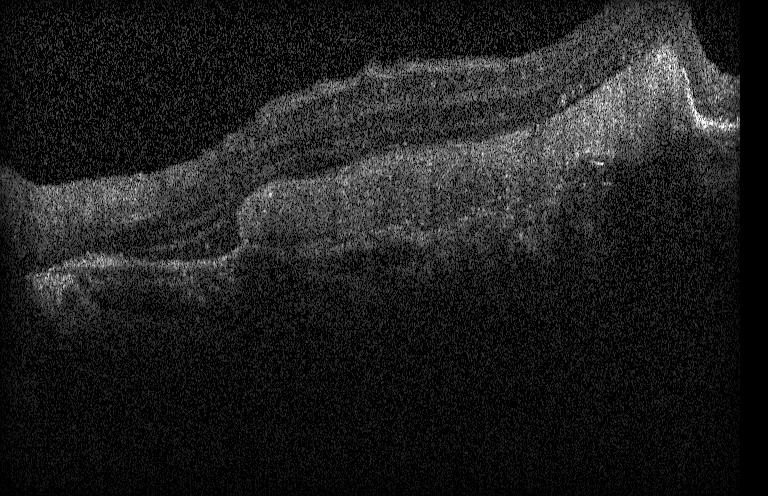

Finding: a choroidal neovascular membrane.